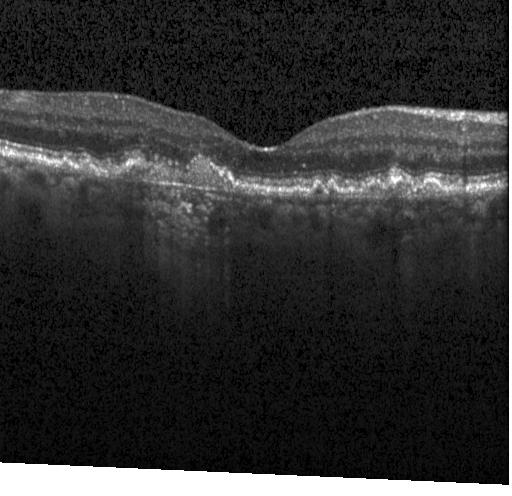

SD-OCT · macular scan · instrument: Heidelberg Spectralis · retinal OCT B-scan.
Choroidal neovascularization.